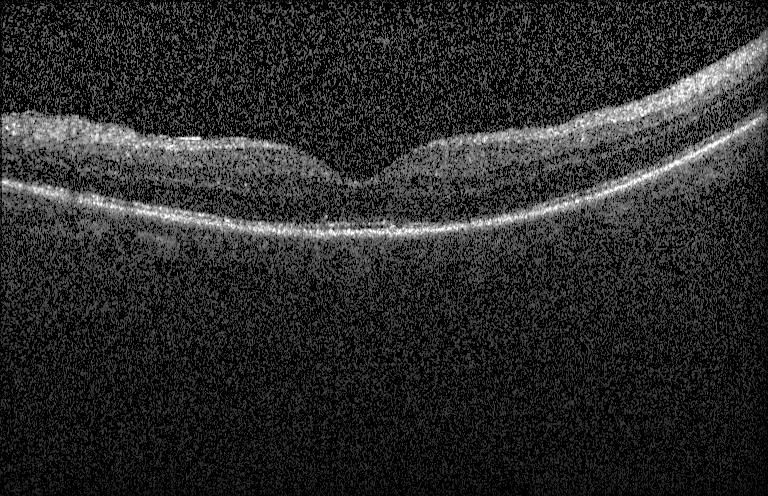 Retinal OCT B-scan, fovea-centered
Impression: no choroidal neovascularization, diabetic macular edema, or drusen.